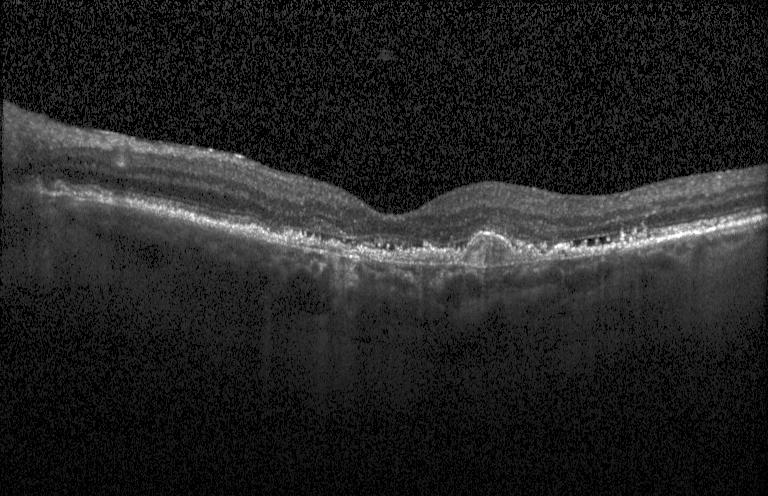

Optical coherence tomography scan — Finding: a choroidal neovascular membrane.